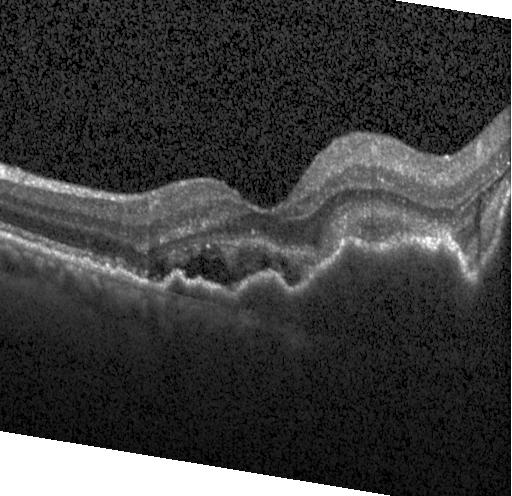 The scan shows choroidal neovascularization.